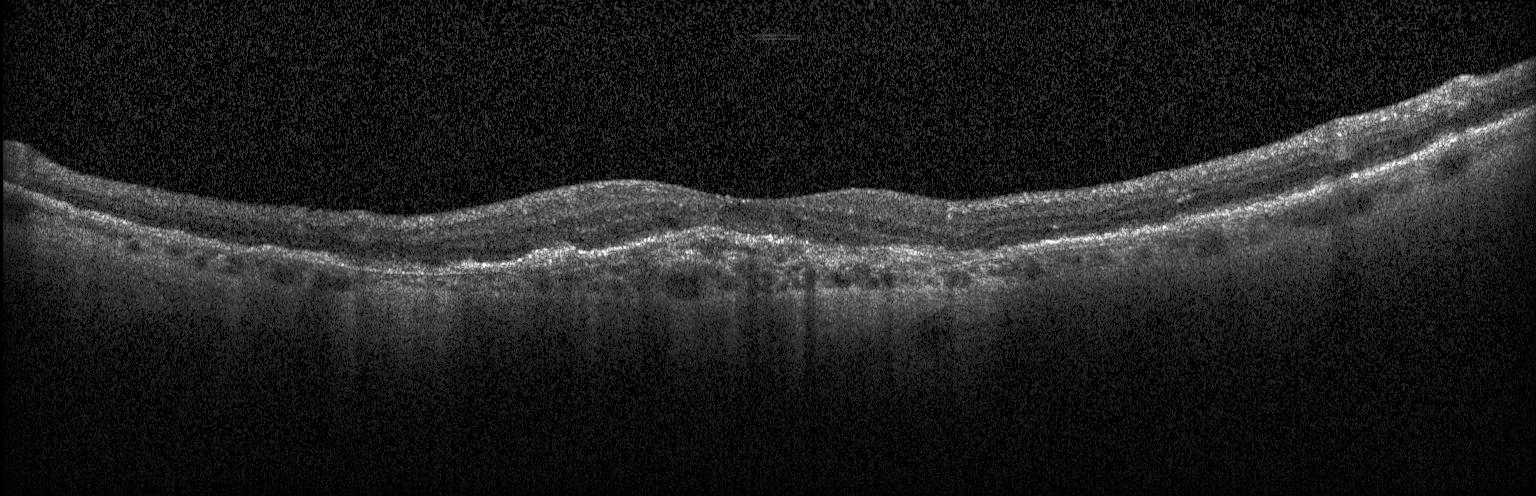
Assessment: choroidal neovascularization.